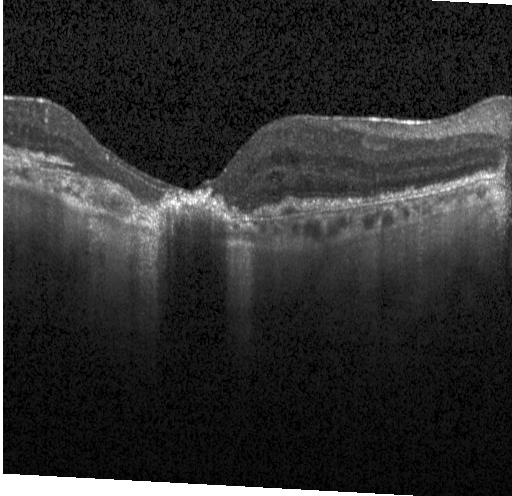 Spectral-domain OCT; instrument: Heidelberg Spectralis; OCT line scan; horizontal scan through the fovea — Finding: choroidal neovascularization.